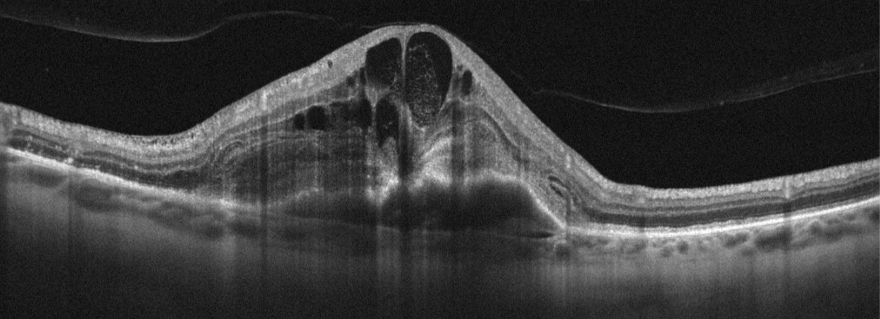 Optovue Avanti RTVue XR · optical coherence tomography B-scan · fovea-centered
Macular OCT: age-related macular degeneration (AMD).